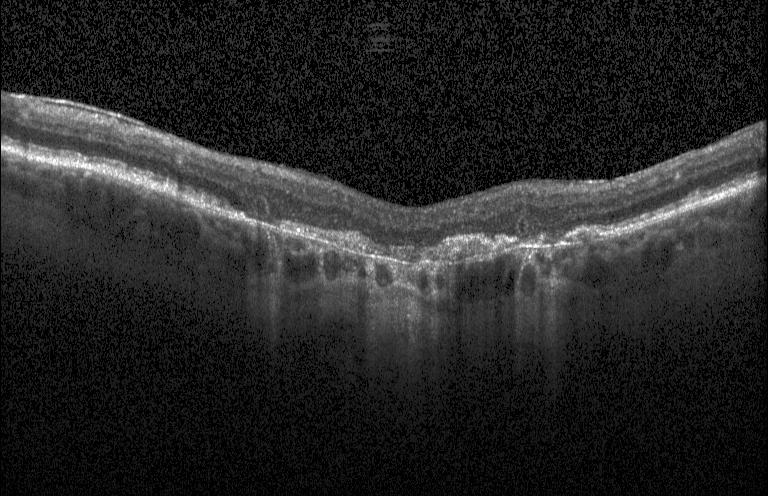

OCT line scan; horizontal scan through the fovea; spectral-domain OCT; Heidelberg Spectralis. Choroidal neovascularization (CNV).